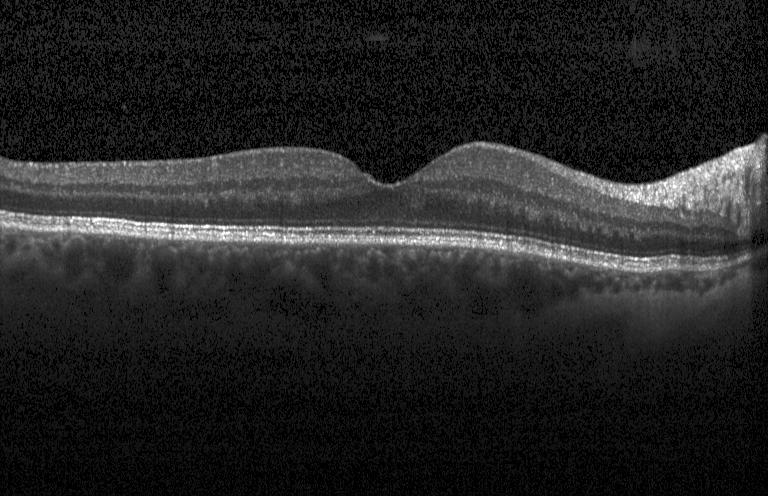

Optical coherence tomography scan, spectral-domain optical coherence tomography. Diagnosis: no choroidal neovascularization, diabetic macular edema, or drusen.